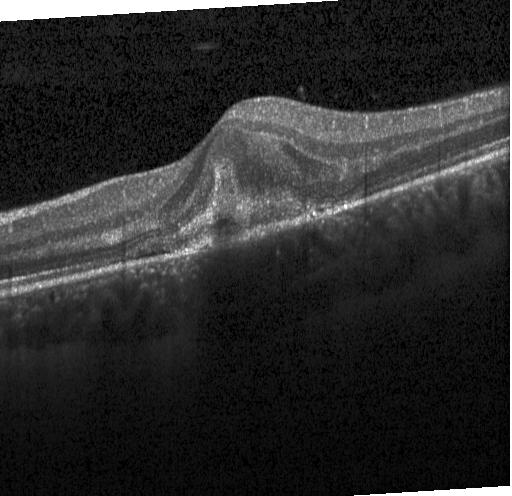

Heidelberg Spectralis OCT system. Retinal OCT B-scan. Spectral-domain OCT.
CNV.